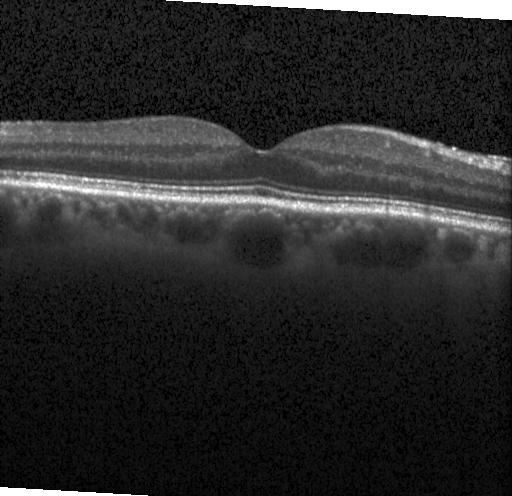 Optical coherence tomography B-scan; instrument: Heidelberg Spectralis.
Finding: neither choroidal neovascularization, diabetic macular edema, nor drusen.